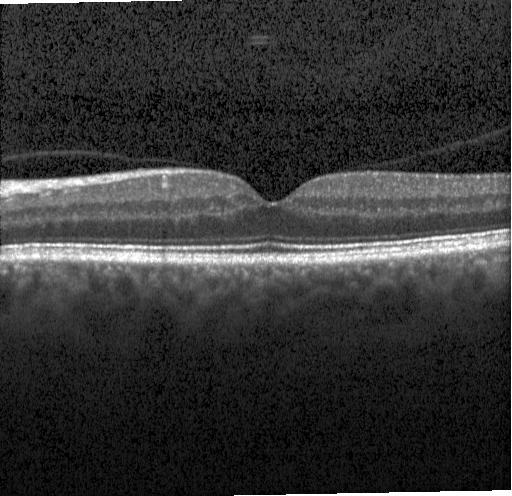
Spectral-domain OCT; retinal OCT B-scan.
Assessment: neither choroidal neovascularization, diabetic macular edema, nor drusen.